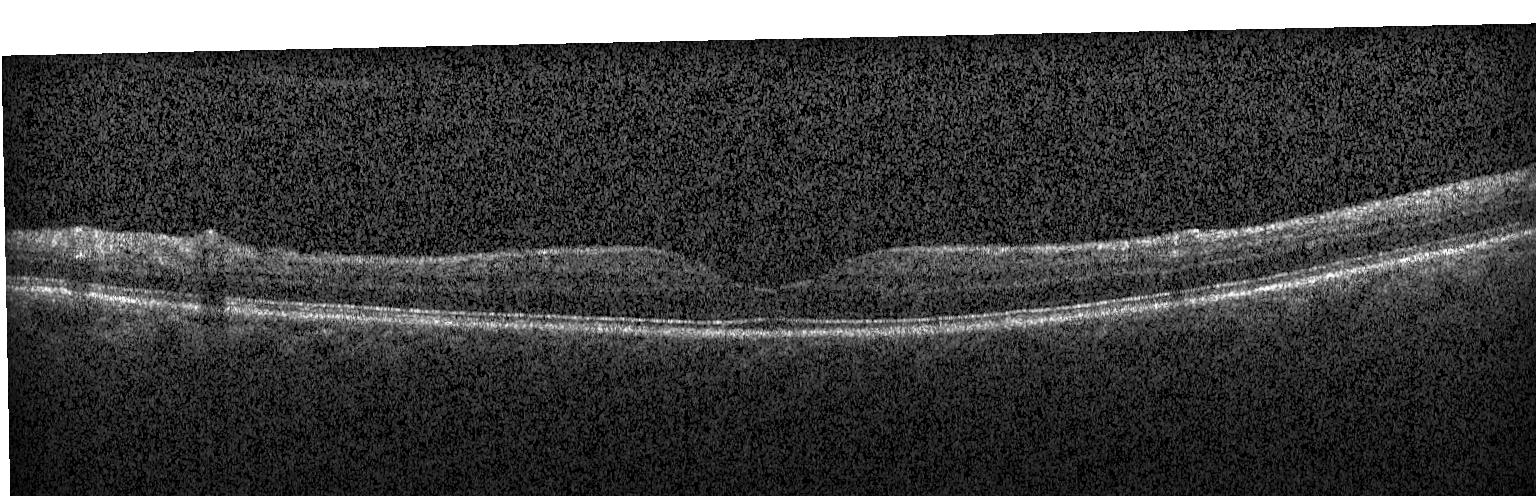

Impression: no evidence of CNV, DME, or drusen.